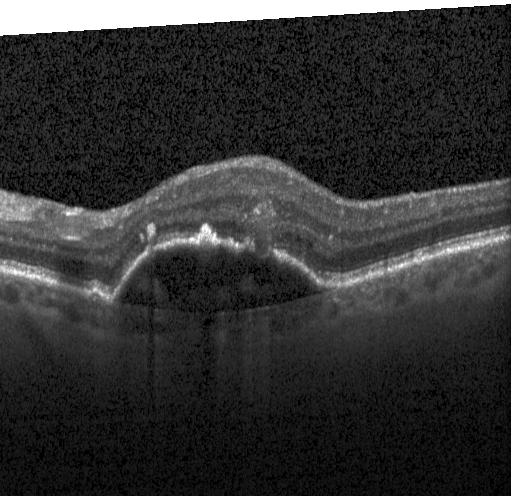

Spectral-domain optical coherence tomography. Optical coherence tomography B-scan. Centered on the fovea. Instrument: Heidelberg Spectralis. Impression: a choroidal neovascular membrane.